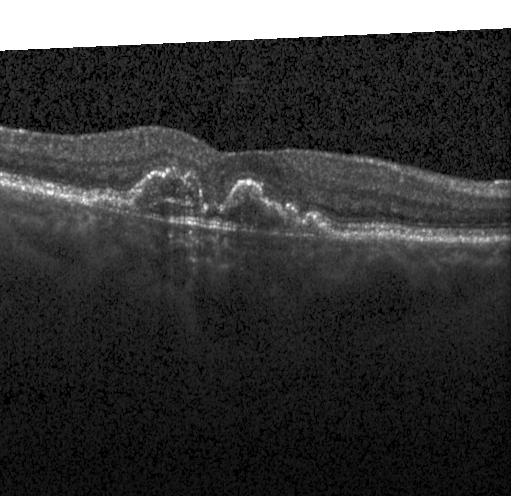 Impression: a choroidal neovascular membrane.